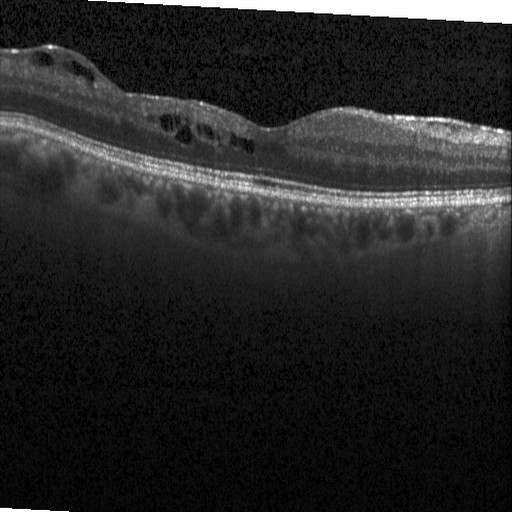 OCT line scan. Diagnosis: DME.